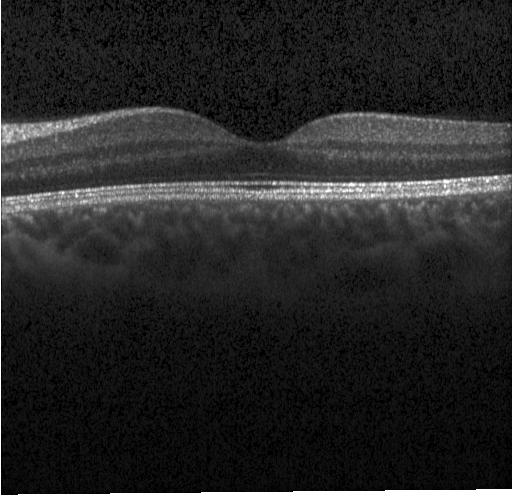
Macular scan, Heidelberg Spectralis OCT system, spectral-domain OCT, OCT B-scan.
This B-scan demonstrates no choroidal neovascularization, diabetic macular edema, or drusen.